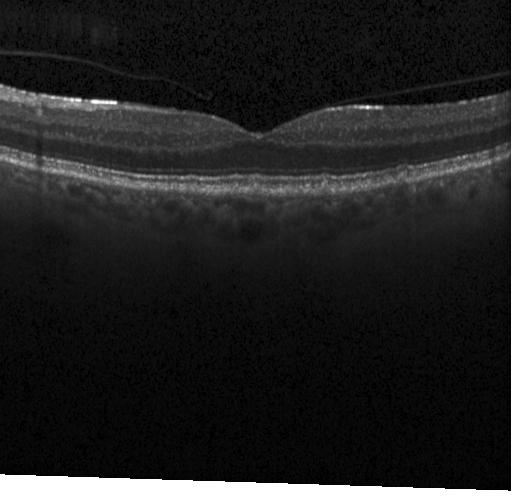

Retinal OCT cross-section showing sub-RPE drusenoid deposits.